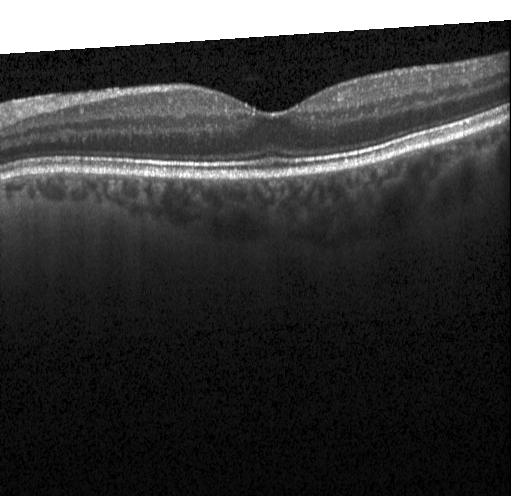

Assessment: no choroidal neovascularization, no diabetic macular edema, and no drusen.